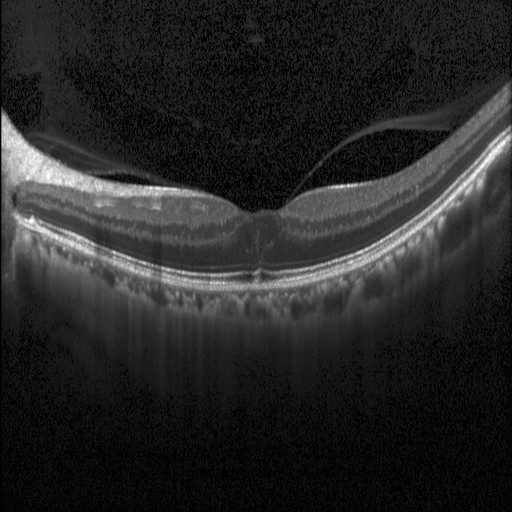

Diabetic macular edema (DME).